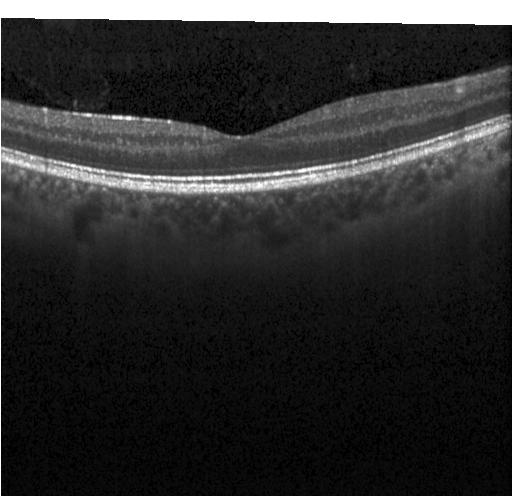
OCT finding: neither CNV, DME, nor drusen.